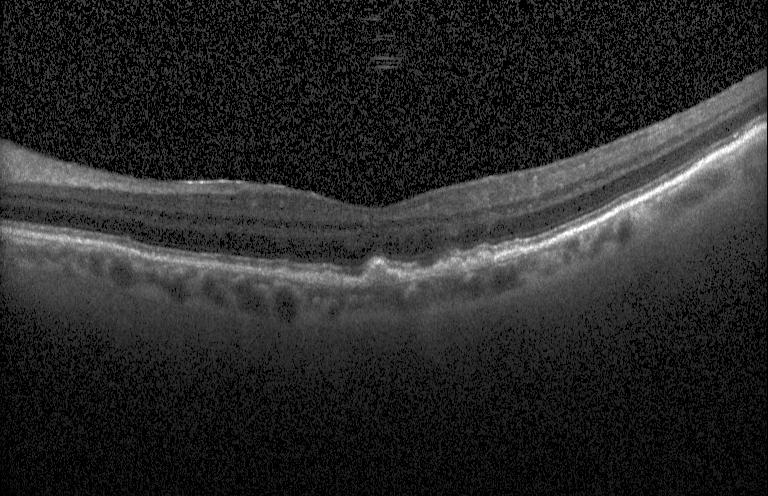

Dx: drusen.